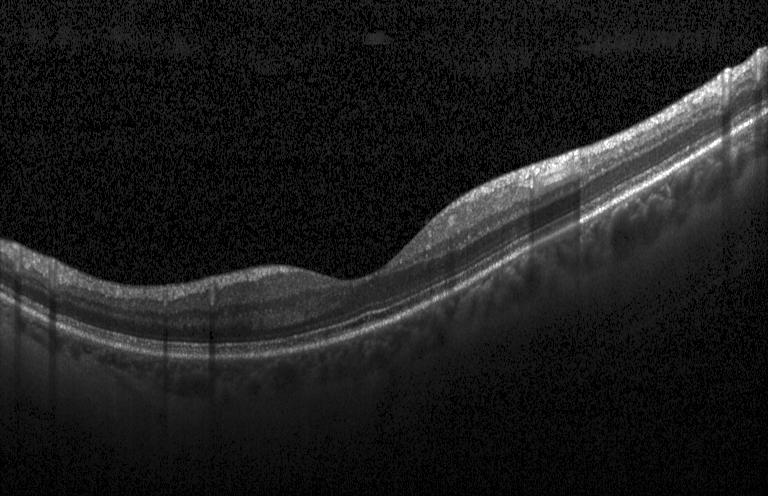

OCT B-scan. Heidelberg Spectralis
No evidence of choroidal neovascularization, diabetic macular edema, or drusen.